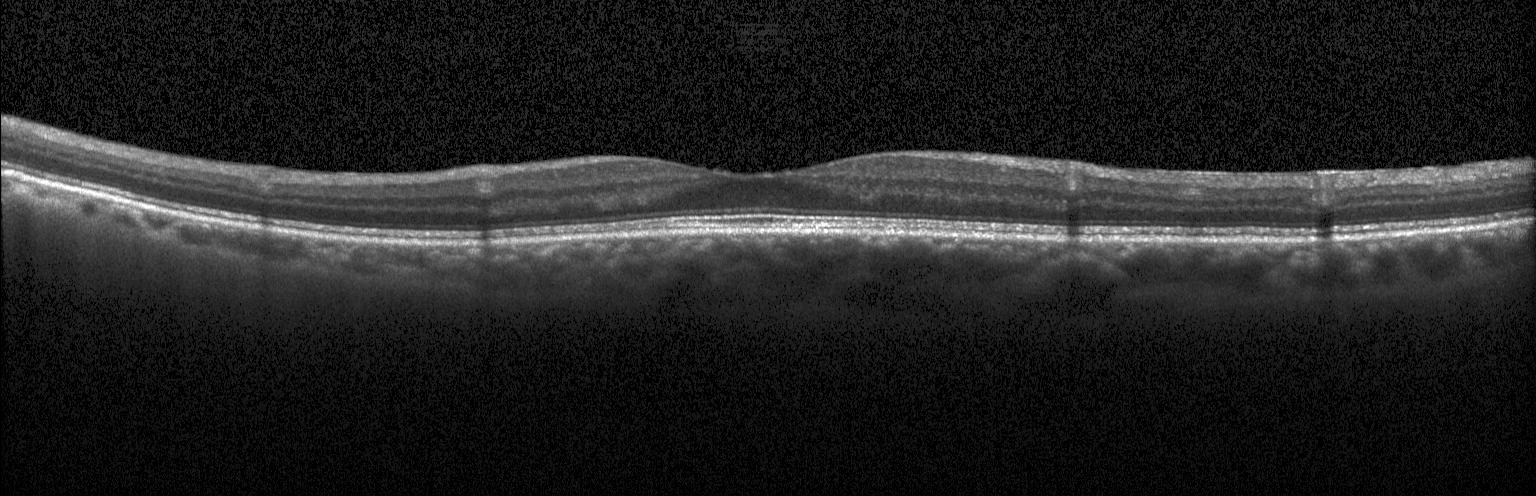
Retinal OCT B-scan. Acquired on a Heidelberg Spectralis. Spectral-domain optical coherence tomography. Through the macula — This B-scan demonstrates neither CNV, DME, nor drusen.